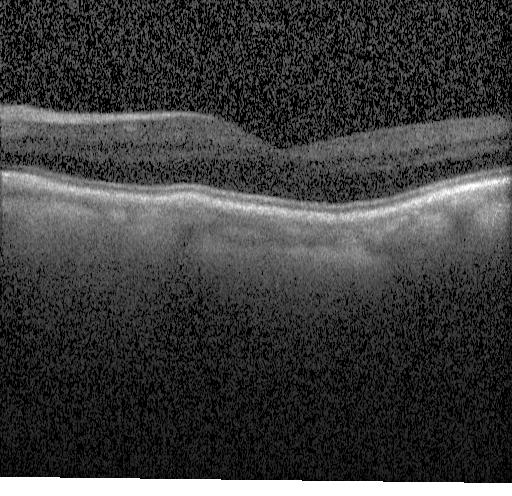

Heidelberg Spectralis · optical coherence tomography B-scan
Macular OCT: no choroidal neovascularization, no diabetic macular edema, and no drusen.